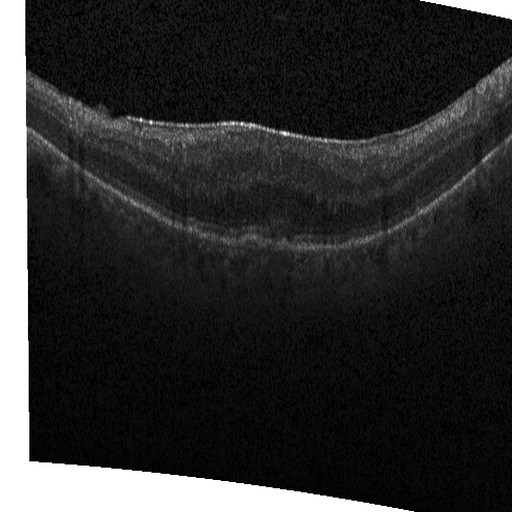

SD-OCT, retinal OCT cross-section, through the macula, acquired on a Heidelberg Spectralis. Impression: diabetic macular edema (DME).